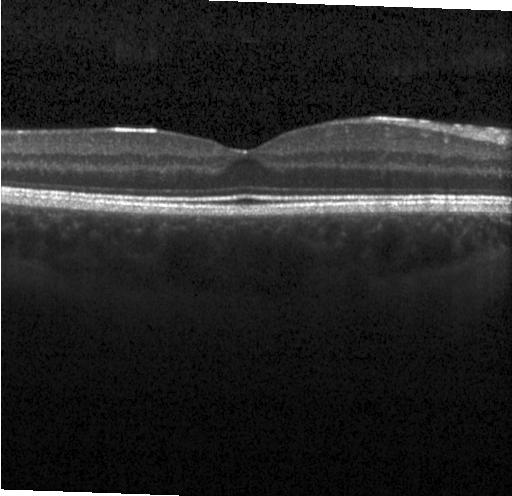

Centered on the fovea. Heidelberg Spectralis. Optical coherence tomography scan. SD-OCT
Impression: no CNV, no DME, and no drusen.